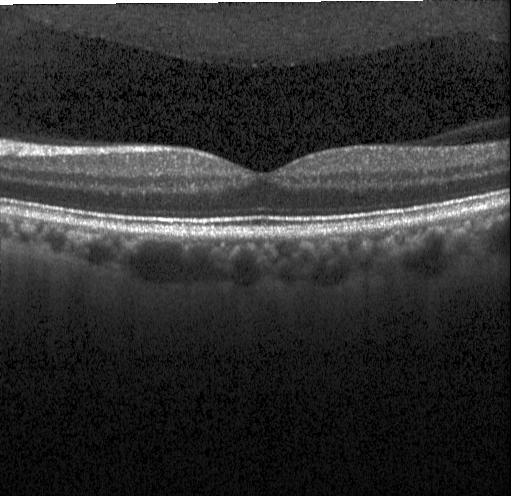 Instrument: Heidelberg Spectralis, spectral-domain OCT, fovea-centered, retinal OCT cross-section
No choroidal neovascularization, no diabetic macular edema, and no drusen.